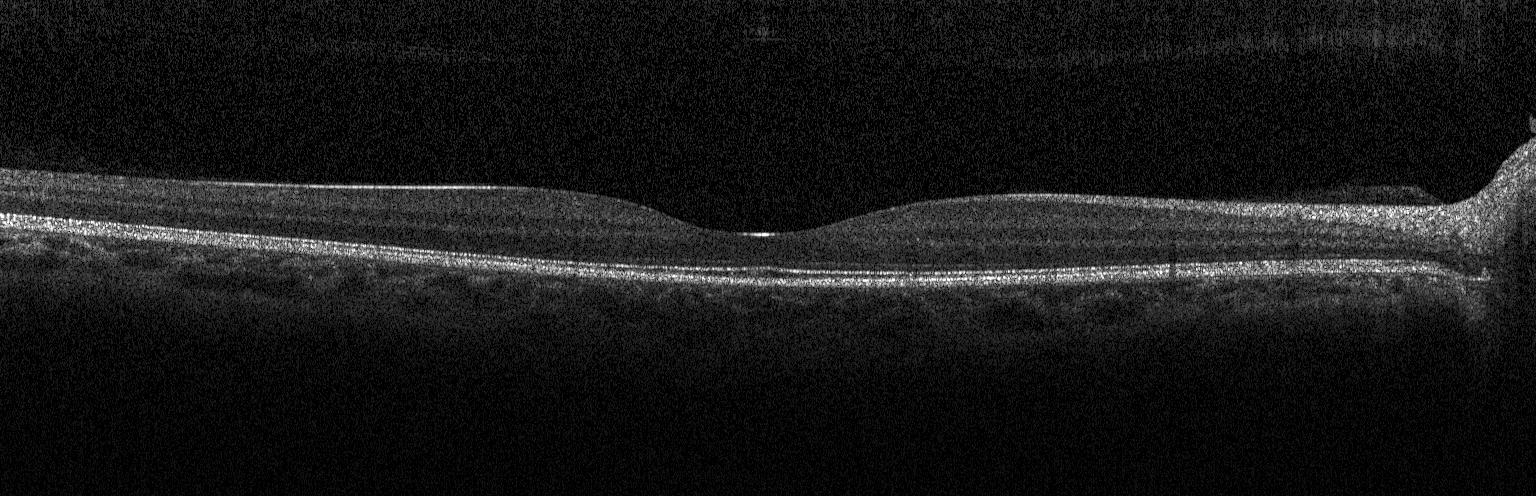 Retinal OCT B-scan. Heidelberg Spectralis OCT system. Spectral-domain OCT
Finding: no CNV, DME, or drusen.